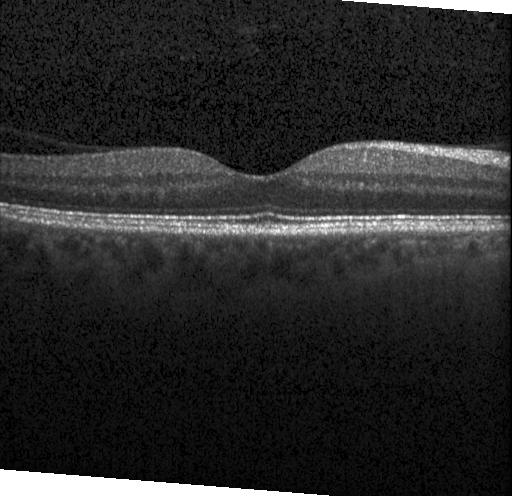 Spectral-domain OCT. Heidelberg Spectralis. OCT line scan.
Diagnosis: no choroidal neovascularization, diabetic macular edema, or drusen.